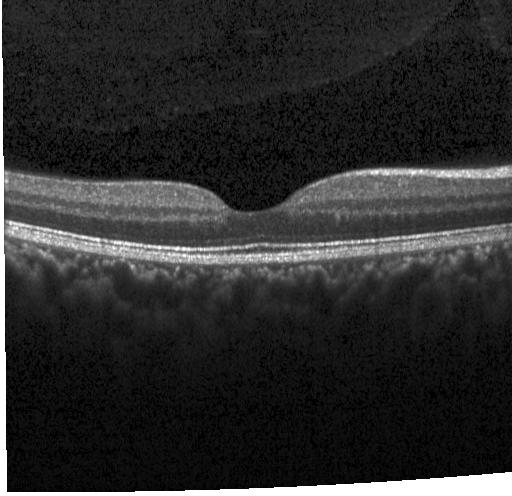 Optical coherence tomography B-scan.
Diagnosis: no evidence of CNV, DME, or drusen.